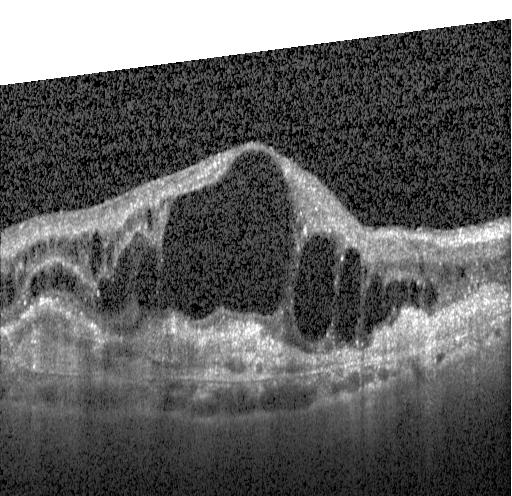 Diagnosis: a choroidal neovascular membrane.